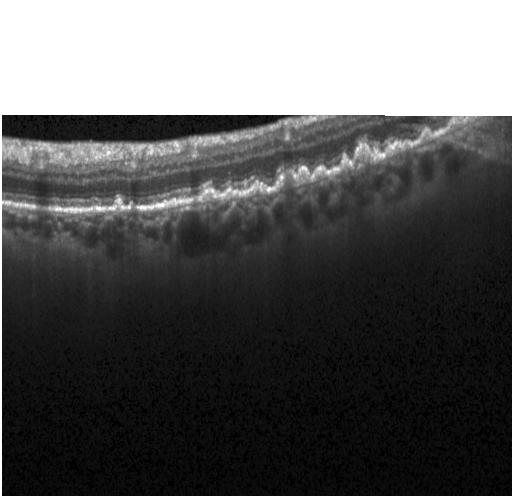 Centered on the fovea. Spectral-domain optical coherence tomography. Retinal OCT B-scan
Diagnosis: multiple drusen.